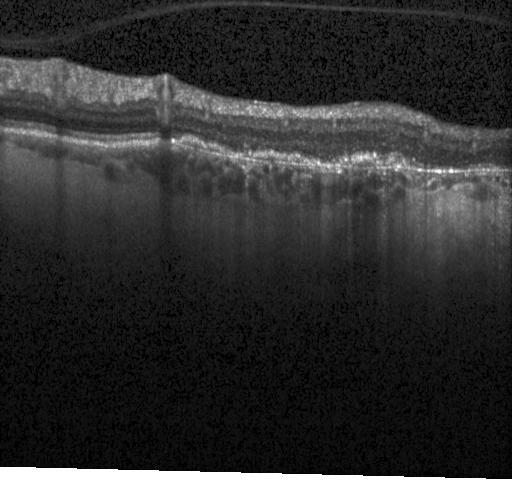 Retinal OCT cross-section, spectral-domain optical coherence tomography, Heidelberg Spectralis OCT system. Assessment: a choroidal neovascular membrane.